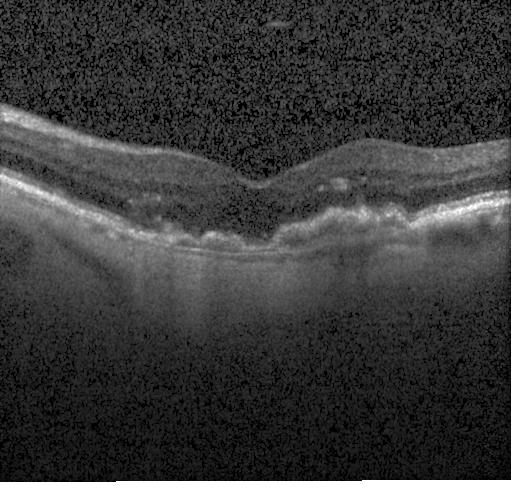
Optical coherence tomography B-scan, spectral-domain OCT — The scan shows CNV.